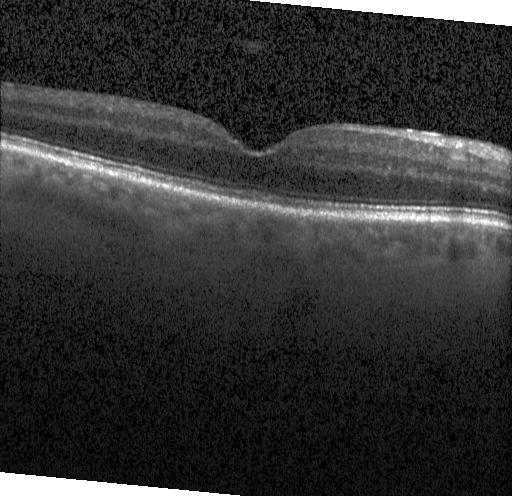 The scan shows neither choroidal neovascularization, diabetic macular edema, nor drusen.